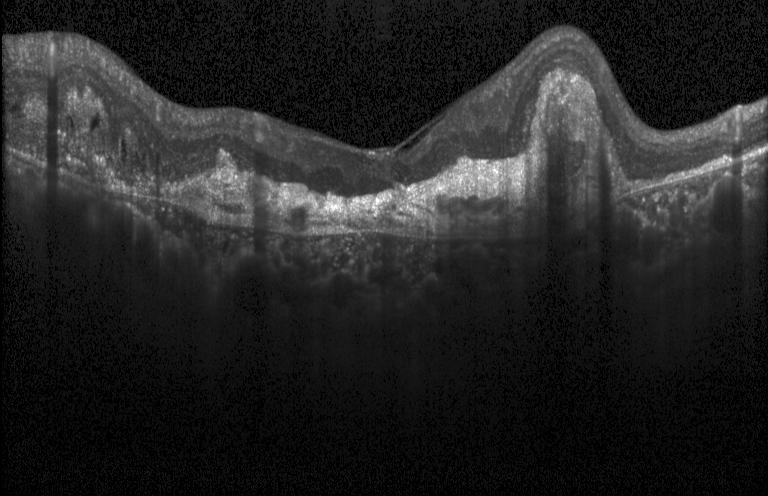 Optical coherence tomography B-scan — Choroidal neovascularization.